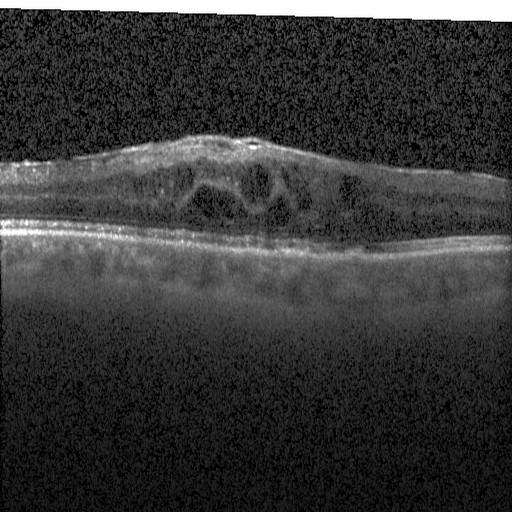 Optical coherence tomography scan.
The scan shows DME.